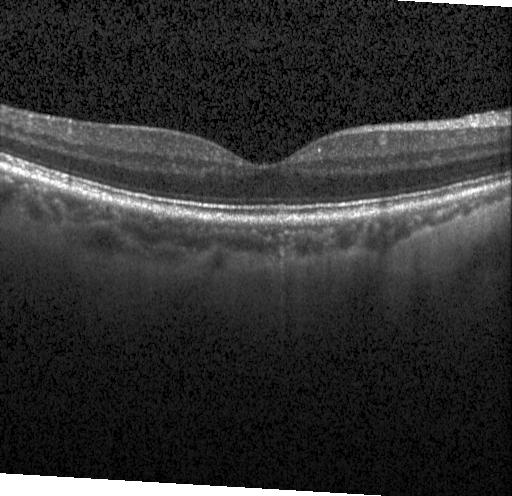

Retinal OCT cross-section · Heidelberg Spectralis · fovea-centered. Impression: no choroidal neovascularization, diabetic macular edema, or drusen.